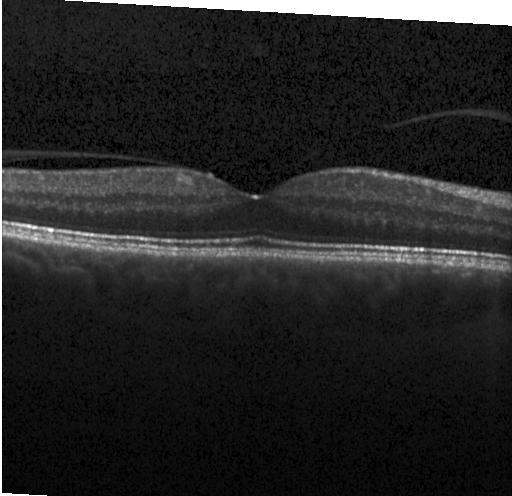
OCT B-scan — Impression: no evidence of choroidal neovascularization, diabetic macular edema, or drusen.